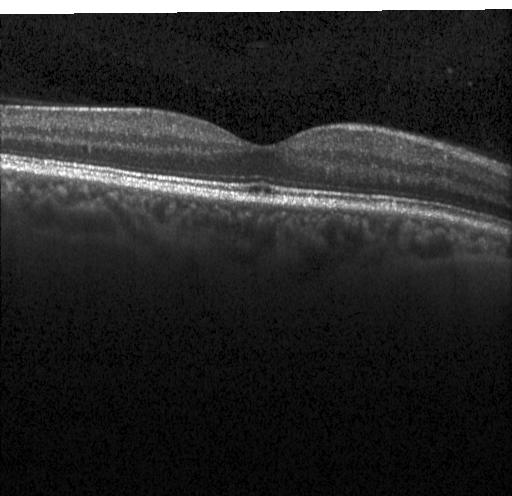
Spectral-domain OCT · Heidelberg Spectralis · retinal OCT cross-section.
Dx: neither choroidal neovascularization, diabetic macular edema, nor drusen.